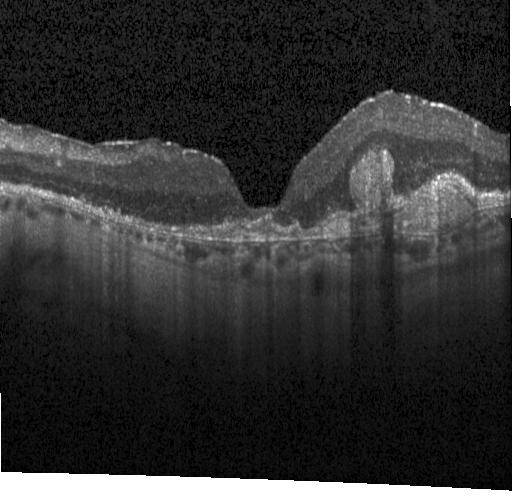 Macular OCT demonstrating a choroidal neovascular membrane.